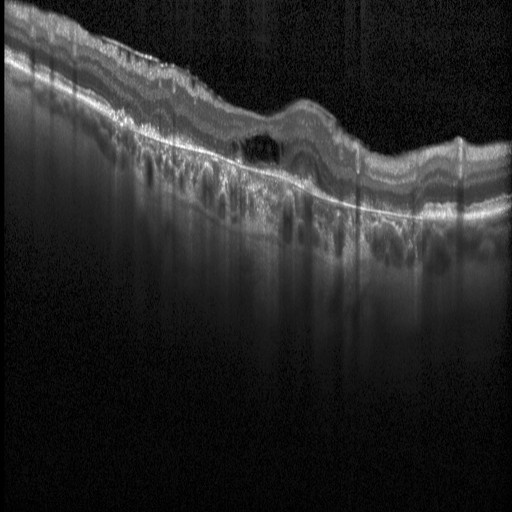

Spectral-domain optical coherence tomography; Heidelberg Spectralis OCT system; optical coherence tomography scan; centered on the fovea. Finding: diabetic macular edema (DME).